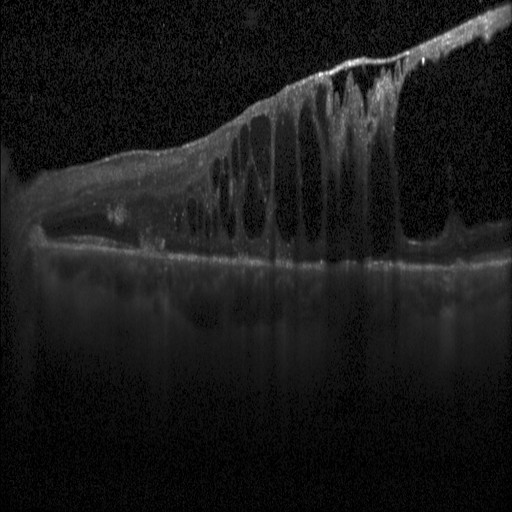
Retinal OCT cross-section — The scan shows diabetic macular edema (DME).